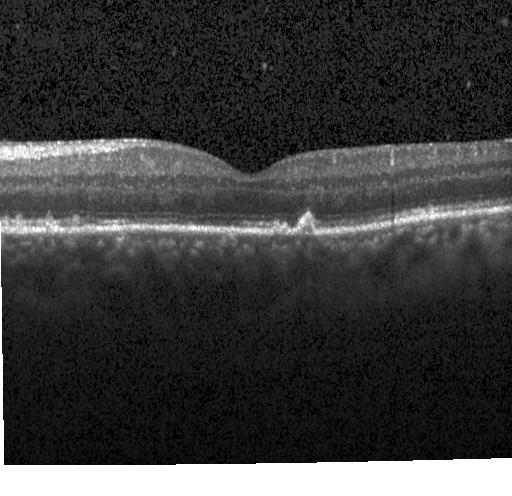

Retinal OCT B-scan.
Impression: drusen.